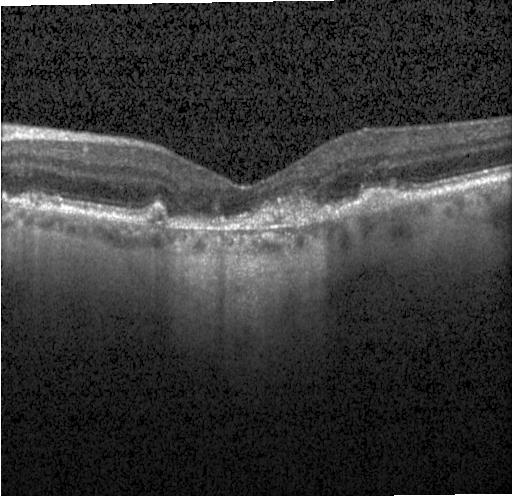 The scan shows CNV.